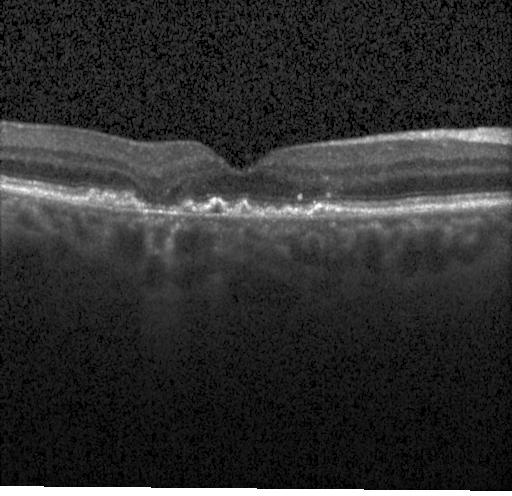
Retinal OCT B-scan — Dx: a choroidal neovascular membrane.